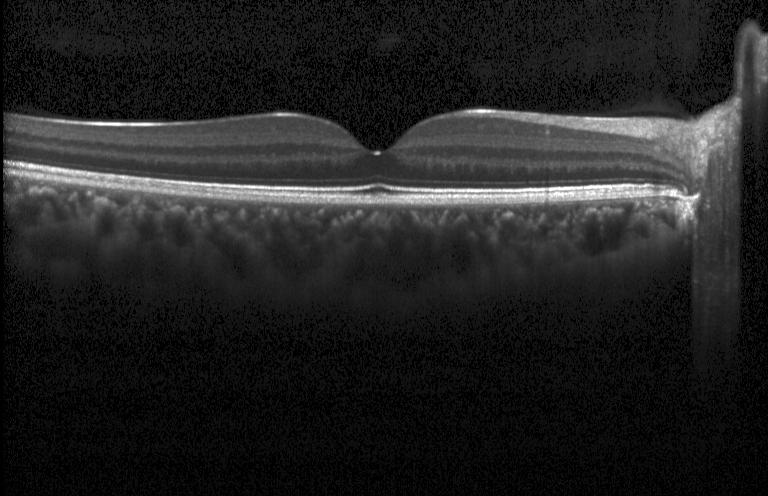
SD-OCT. Optical coherence tomography scan
Dx: no choroidal neovascularization, no diabetic macular edema, and no drusen.